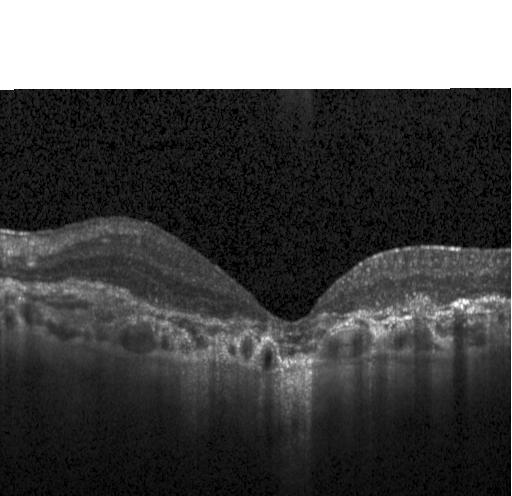

Retinal OCT cross-section — Assessment: a choroidal neovascular membrane.